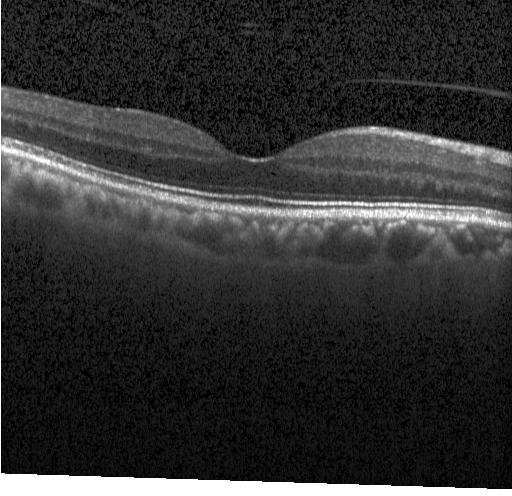 Macular OCT demonstrating neither choroidal neovascularization, diabetic macular edema, nor drusen.